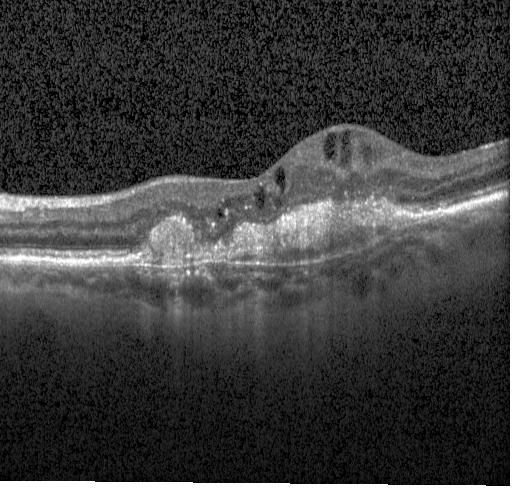 Through the macula · retinal OCT B-scan · SD-OCT · instrument: Heidelberg Spectralis.
Macular OCT: a choroidal neovascular membrane.